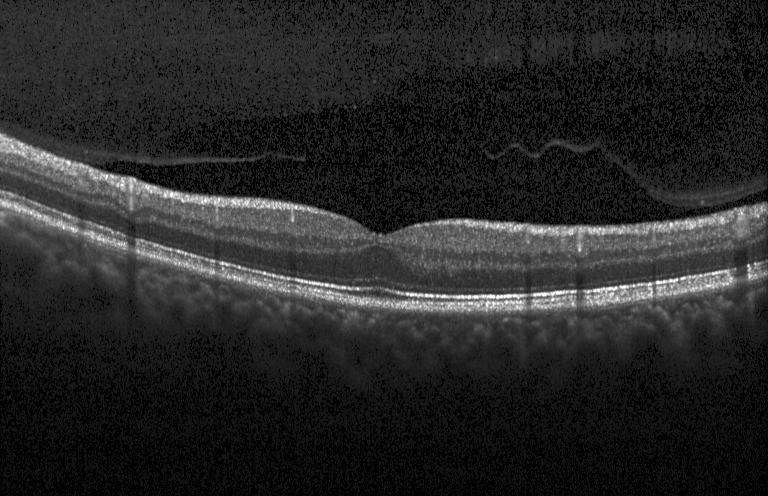
Instrument: Heidelberg Spectralis. SD-OCT. Macular scan. OCT line scan
Assessment: no choroidal neovascularization, diabetic macular edema, or drusen.